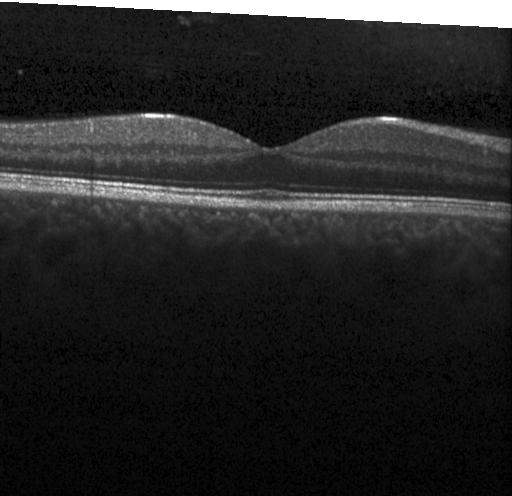 Diagnosis: no evidence of choroidal neovascularization, diabetic macular edema, or drusen.